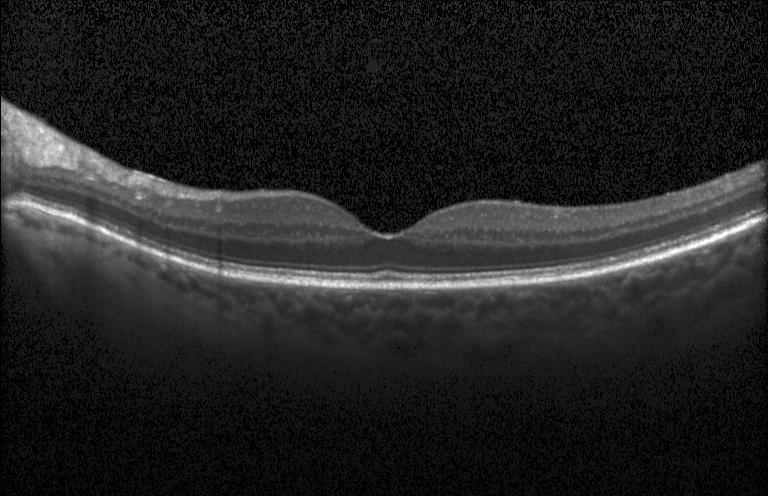
Optical coherence tomography B-scan. No CNV, no DME, and no drusen.